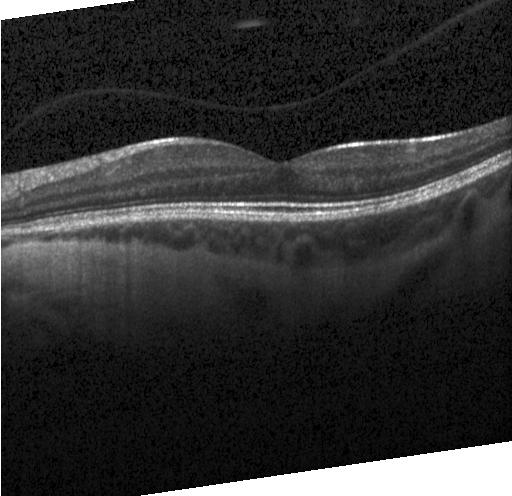

Spectral-domain OCT; retinal OCT B-scan; Heidelberg Spectralis OCT system; through the macula
Diagnosis: no CNV, DME, or drusen.